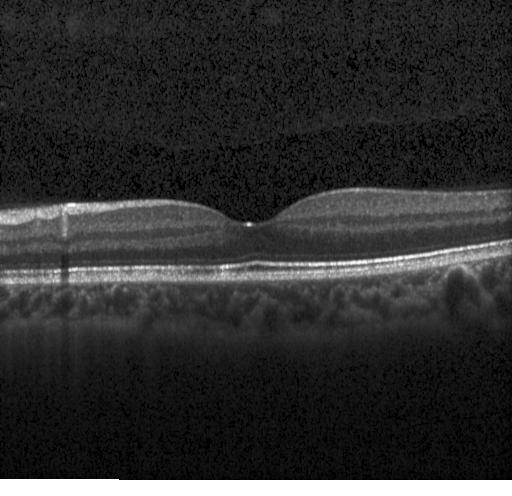

Optical coherence tomography scan — The scan shows no evidence of CNV, DME, or drusen.